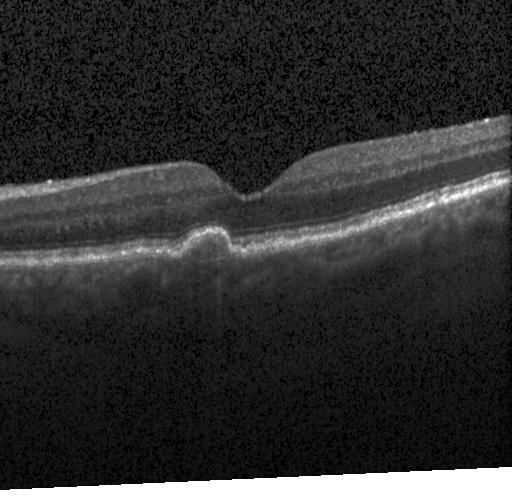 Diagnosis: drusen.